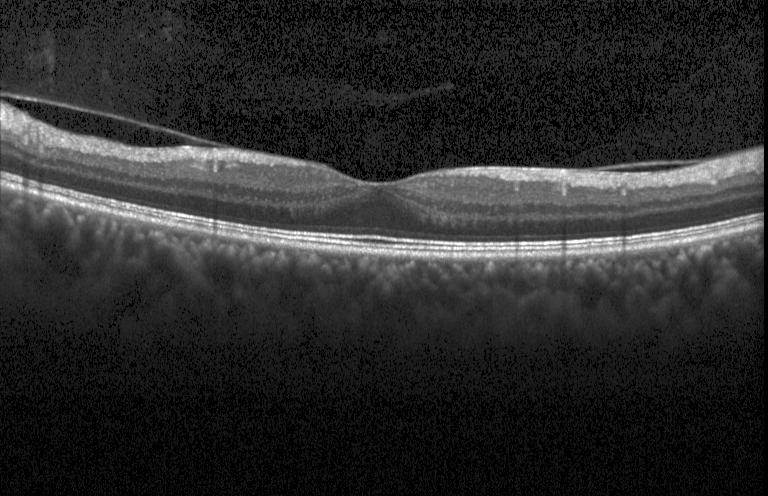
Acquired on a Heidelberg Spectralis; horizontal scan through the fovea; spectral-domain optical coherence tomography; OCT line scan.
The scan shows no choroidal neovascularization, no diabetic macular edema, and no drusen.